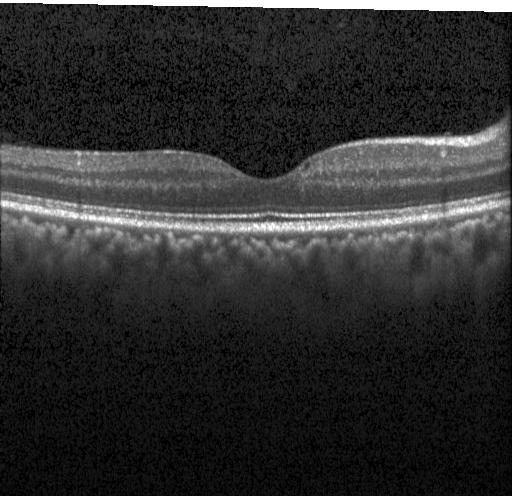
Assessment: no choroidal neovascularization, no diabetic macular edema, and no drusen.